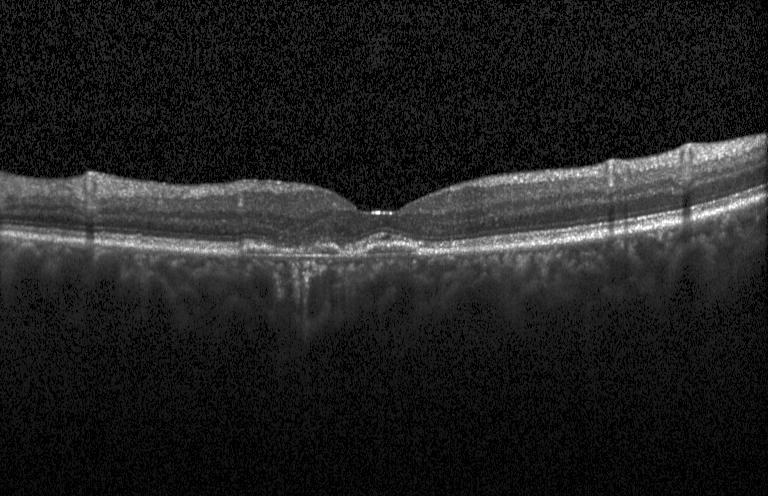
The scan shows a choroidal neovascular membrane.